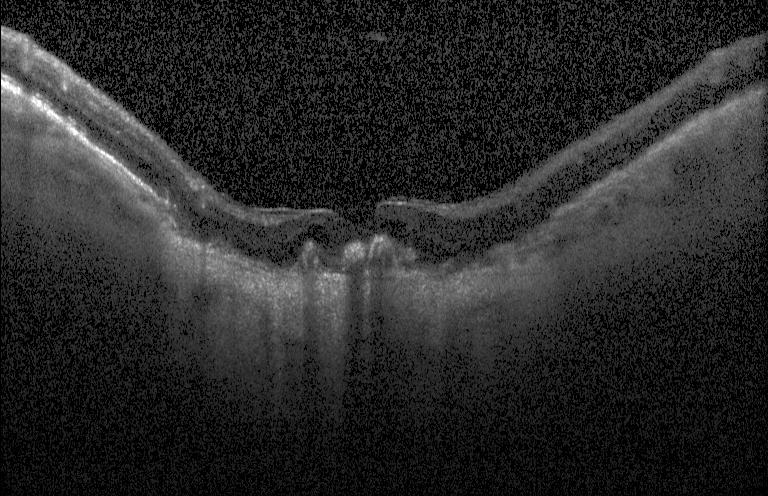 Spectral-domain OCT. OCT B-scan. Acquired on a Heidelberg Spectralis.
Finding: a choroidal neovascular membrane.